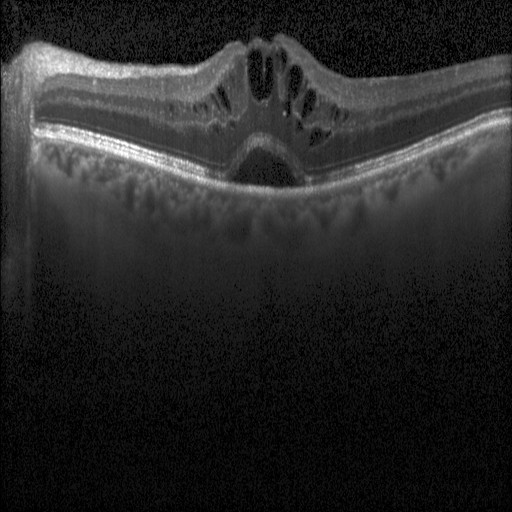
Optical coherence tomography scan.
The scan shows diabetic macular edema (DME).